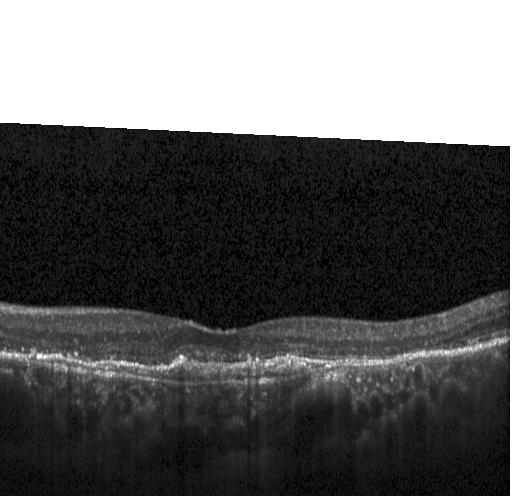
Macular OCT: choroidal neovascularization (CNV).